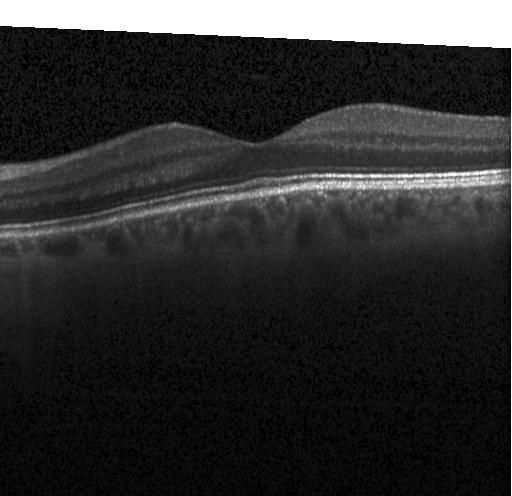 Optical coherence tomography B-scan.
Diagnosis: neither choroidal neovascularization, diabetic macular edema, nor drusen.